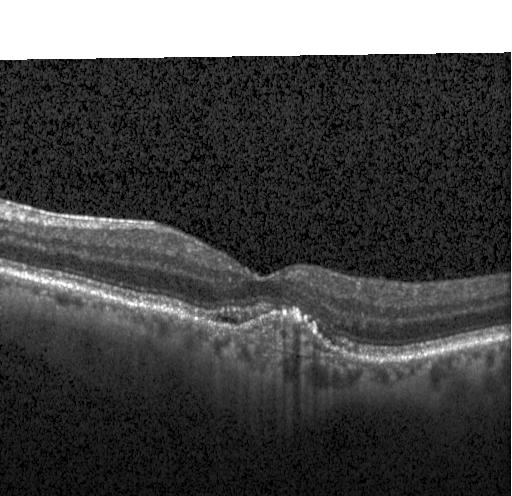

OCT B-scan. Heidelberg Spectralis OCT system. Assessment: choroidal neovascularization.